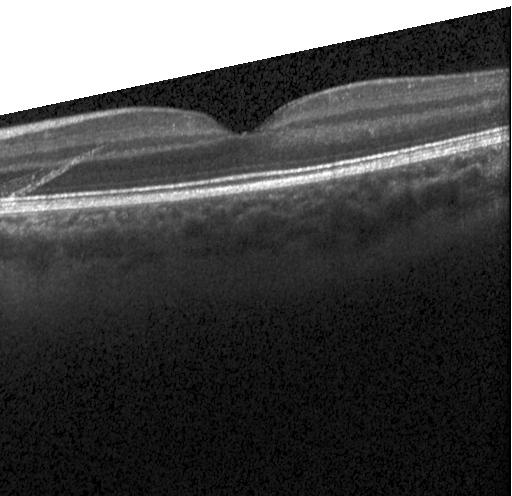
Optical coherence tomography B-scan; acquired on a Heidelberg Spectralis; spectral-domain OCT. Dx: no evidence of choroidal neovascularization, diabetic macular edema, or drusen.